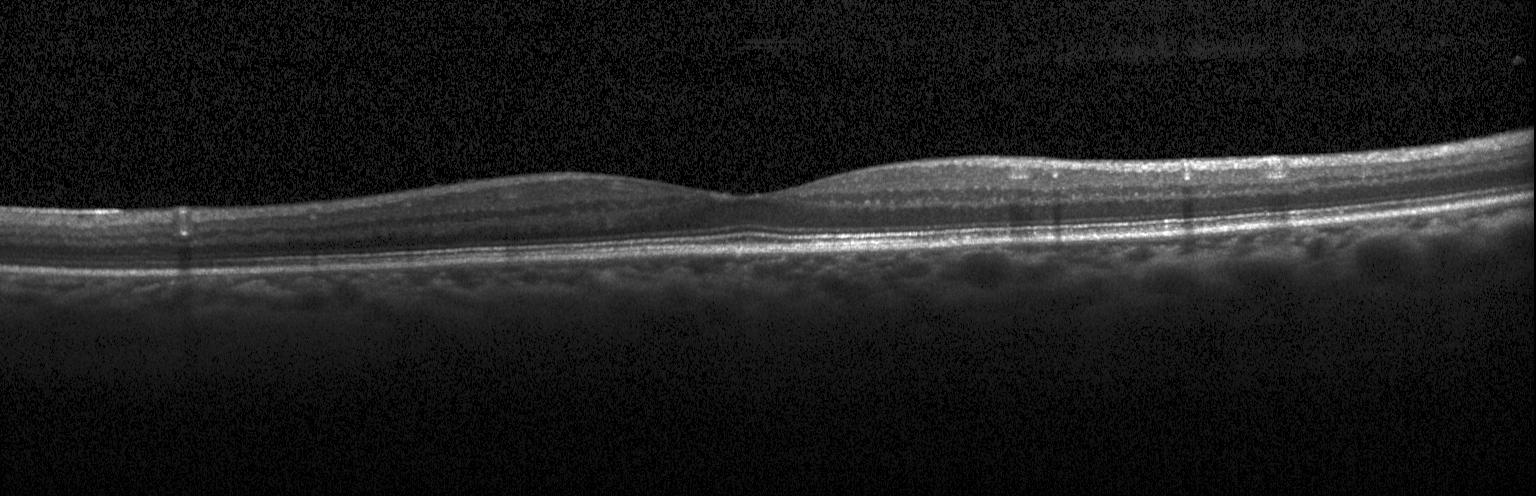

Macular OCT demonstrating no evidence of CNV, DME, or drusen.